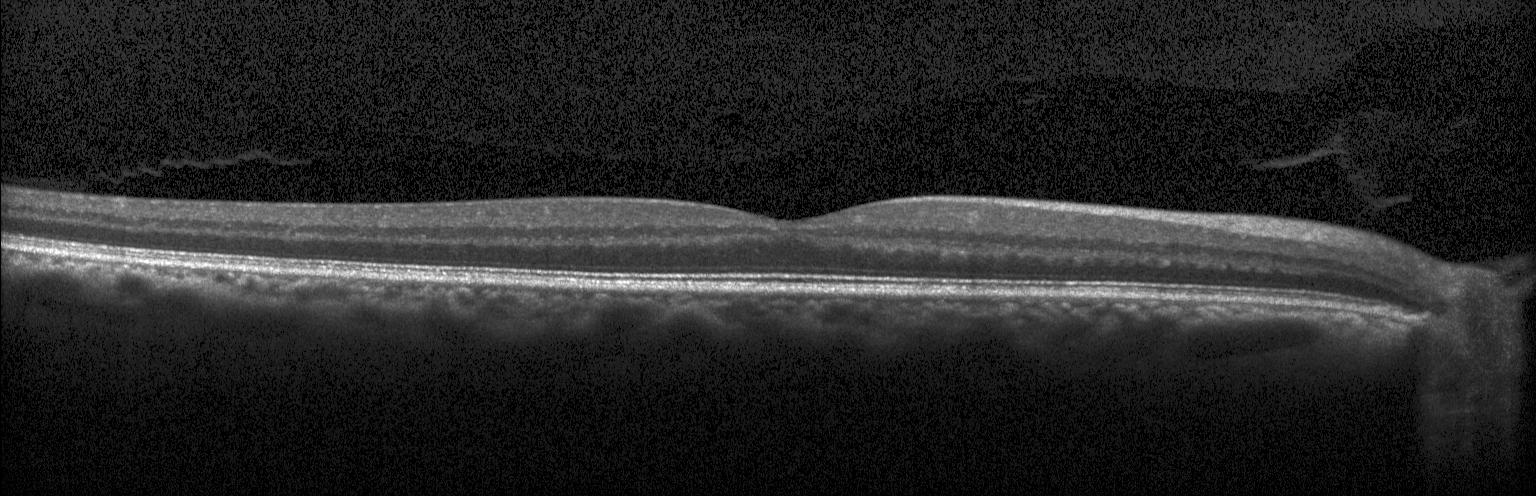
Optical coherence tomography B-scan
Assessment: no choroidal neovascularization, diabetic macular edema, or drusen.